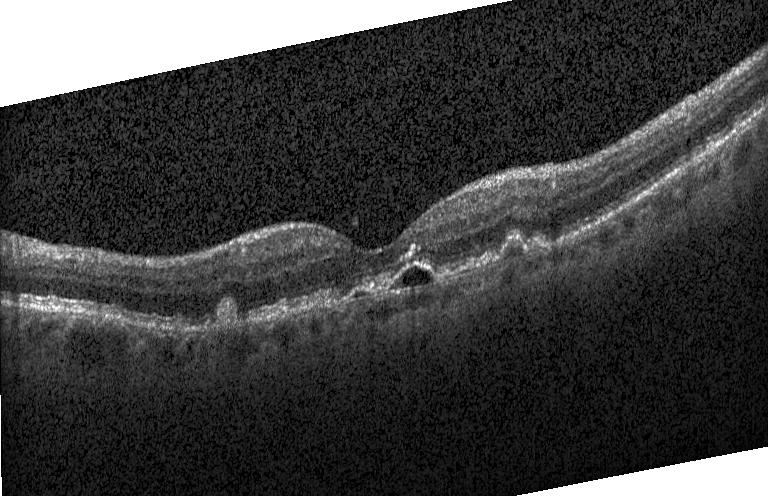

Macular OCT demonstrating choroidal neovascularization (CNV).